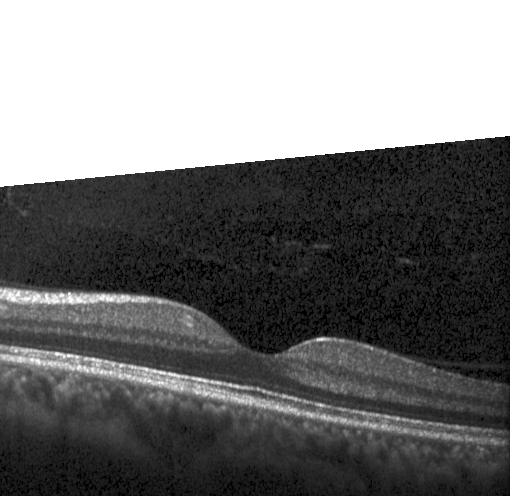
OCT line scan
Macular OCT: neither choroidal neovascularization, diabetic macular edema, nor drusen.